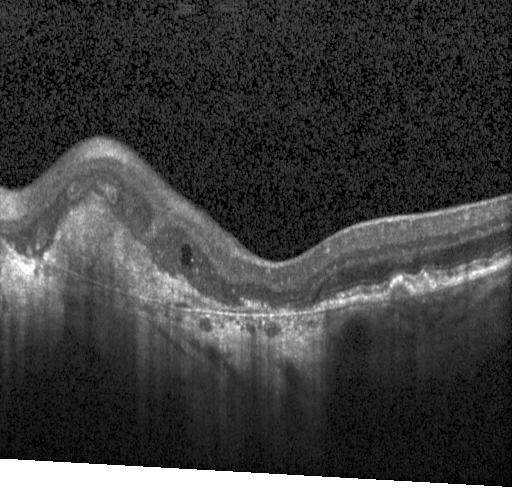
Spectral-domain optical coherence tomography; macular scan; Heidelberg Spectralis OCT system; OCT line scan.
Impression: CNV.